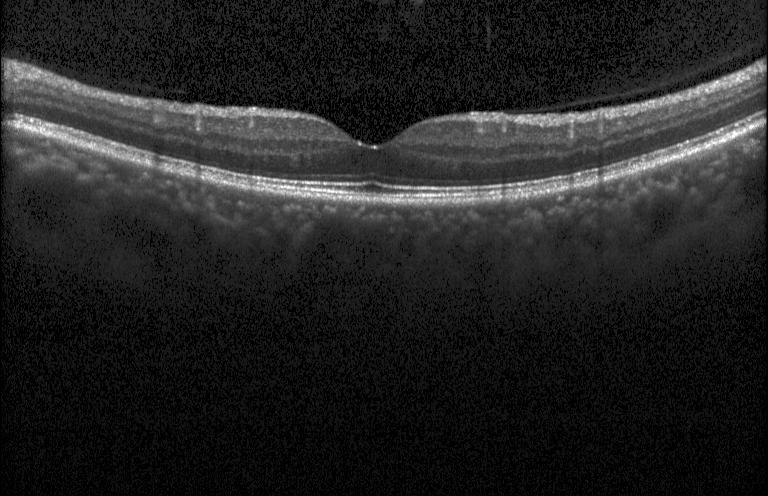 Macular OCT demonstrating no evidence of CNV, DME, or drusen.